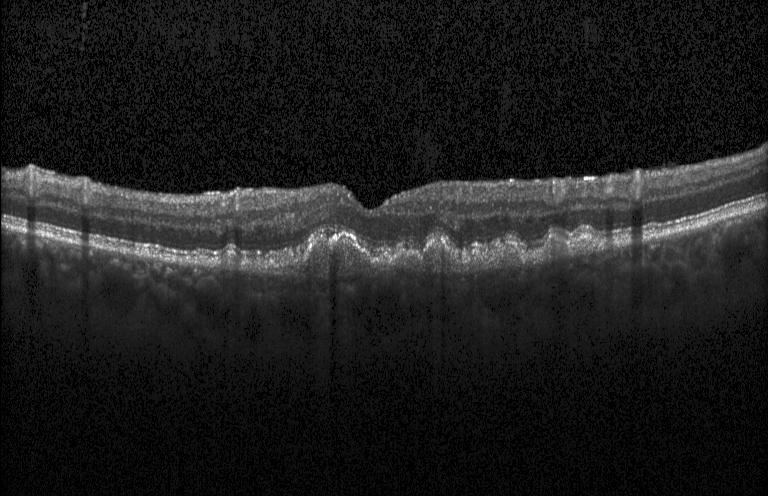

OCT B-scan. Through the macula. Heidelberg Spectralis OCT system. Spectral-domain OCT. Dx: choroidal neovascularization (CNV).